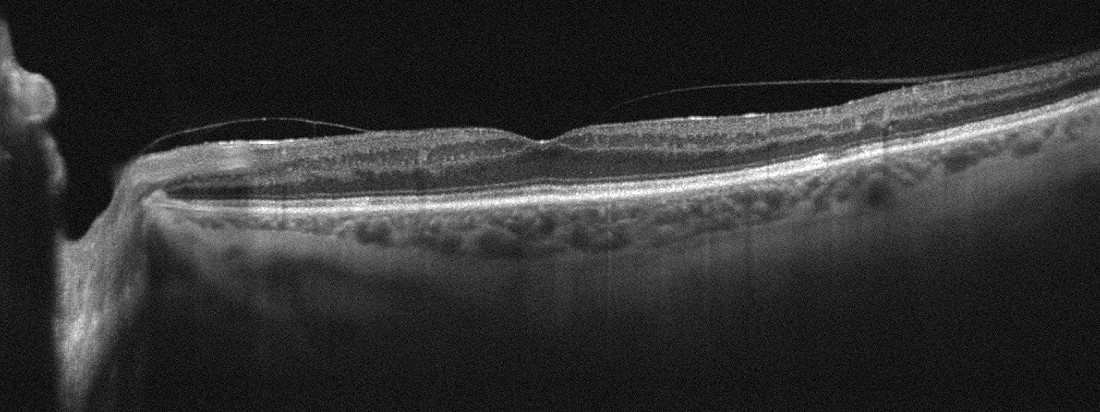
Acquired on an Optovue Avanti RTVue XR, through the macula, optical coherence tomography scan.
The scan shows diabetic macular edema (DME).